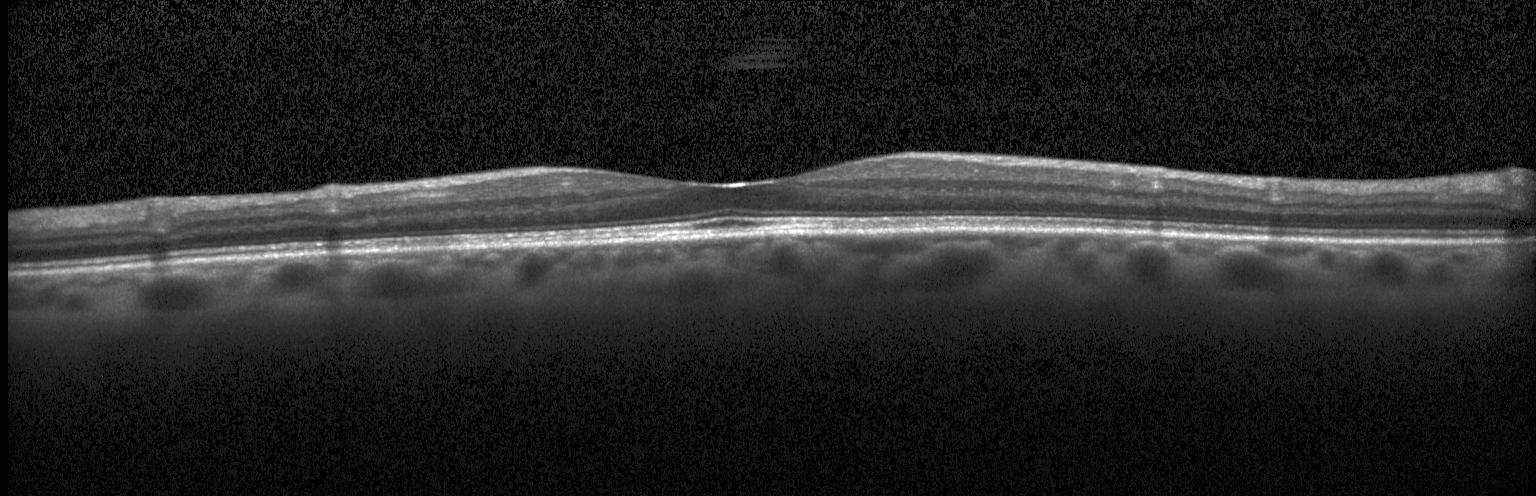

OCT B-scan; instrument: Heidelberg Spectralis; spectral-domain OCT; macular scan — Diagnosis: no choroidal neovascularization, no diabetic macular edema, and no drusen.